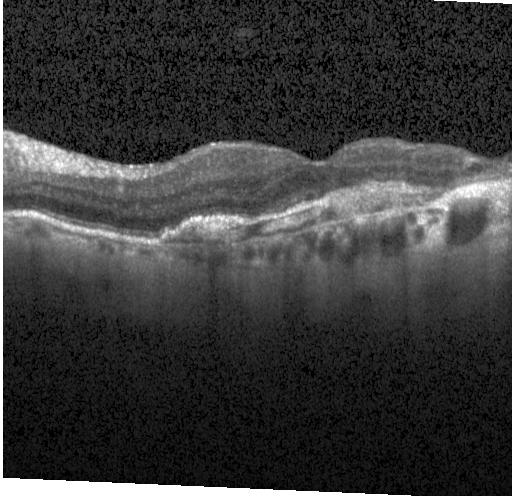

Spectral-domain optical coherence tomography, Heidelberg Spectralis, through the macula, optical coherence tomography scan. Finding: a choroidal neovascular membrane.